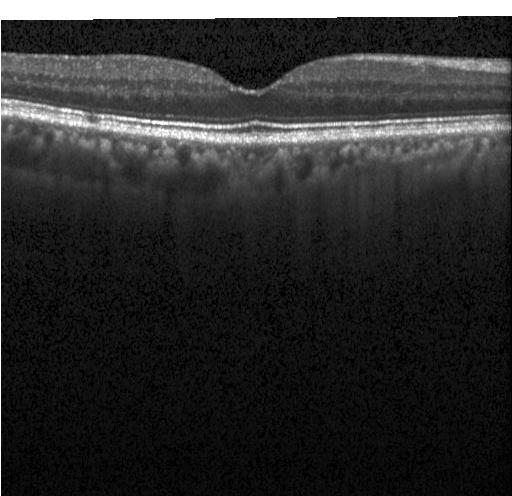
Macular scan. OCT B-scan. Spectral-domain optical coherence tomography. Finding: no evidence of choroidal neovascularization, diabetic macular edema, or drusen.